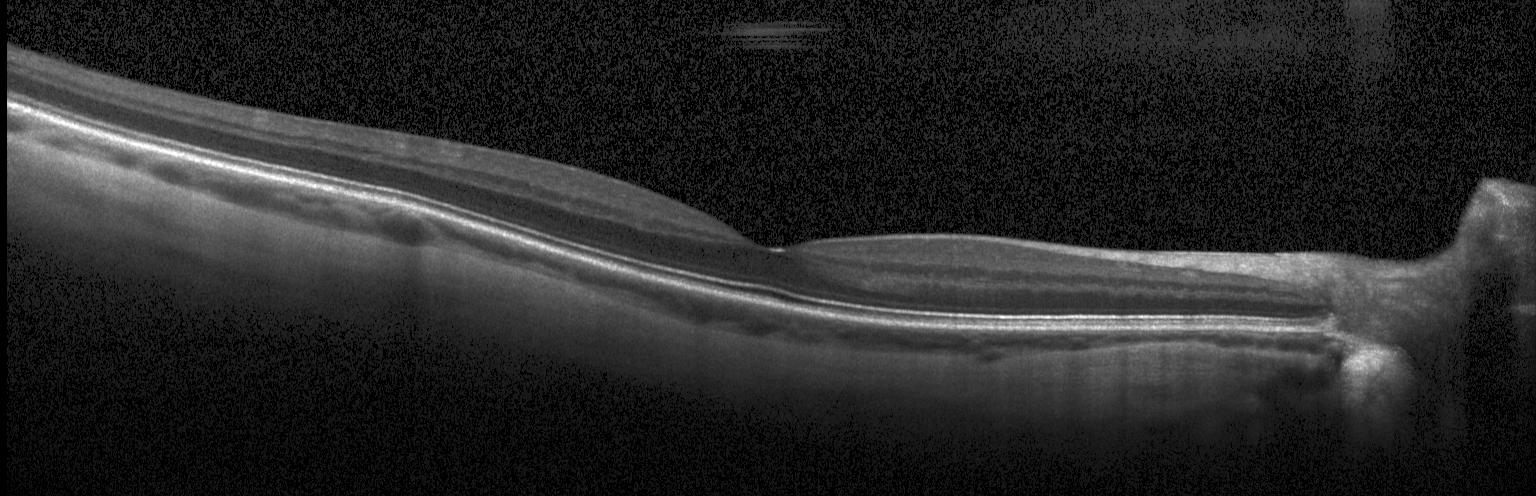

Retinal OCT cross-section.
Dx: neither choroidal neovascularization, diabetic macular edema, nor drusen.